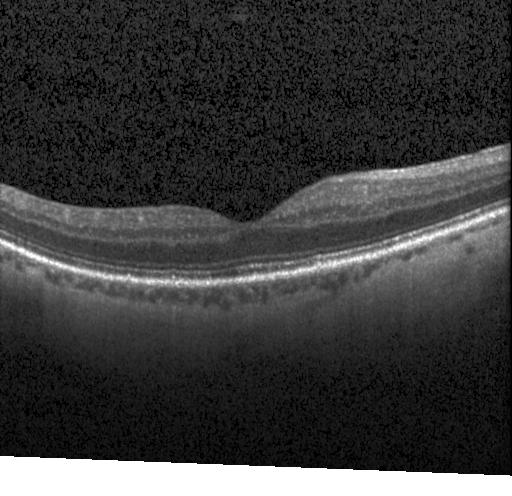 OCT line scan · SD-OCT. Dx: no CNV, DME, or drusen.